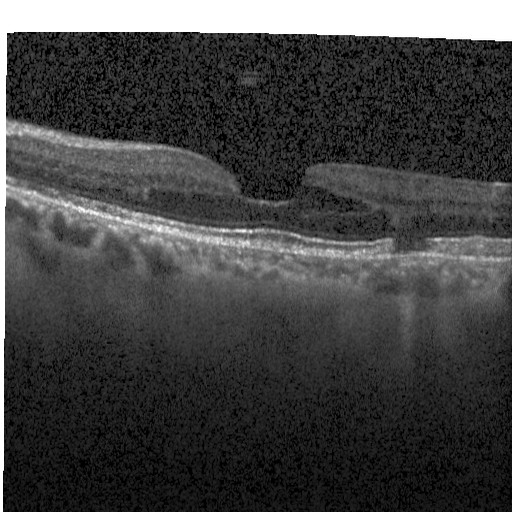 Diagnosis: diabetic macular edema.